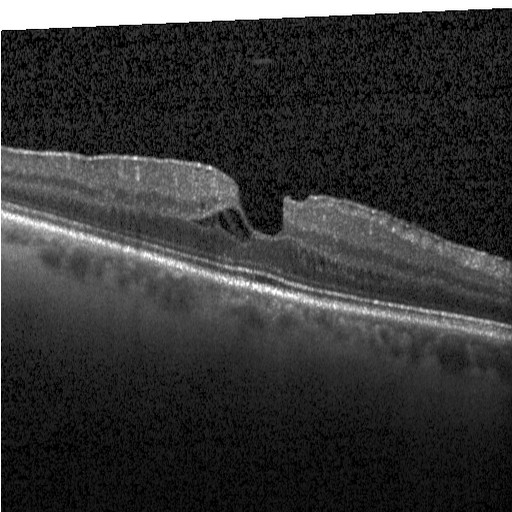

Assessment: diabetic macular edema.